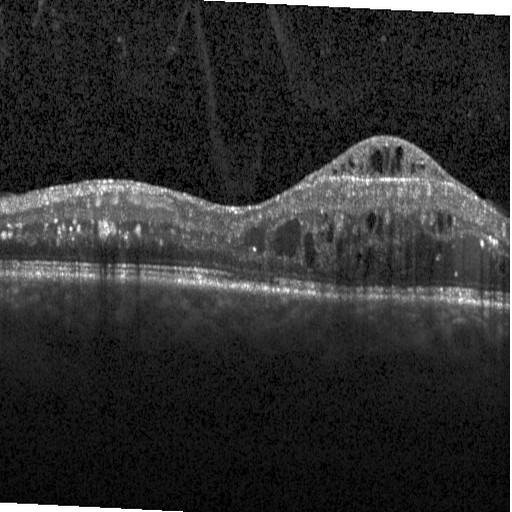
Optical coherence tomography scan — Diagnosis: diabetic macular edema (DME).